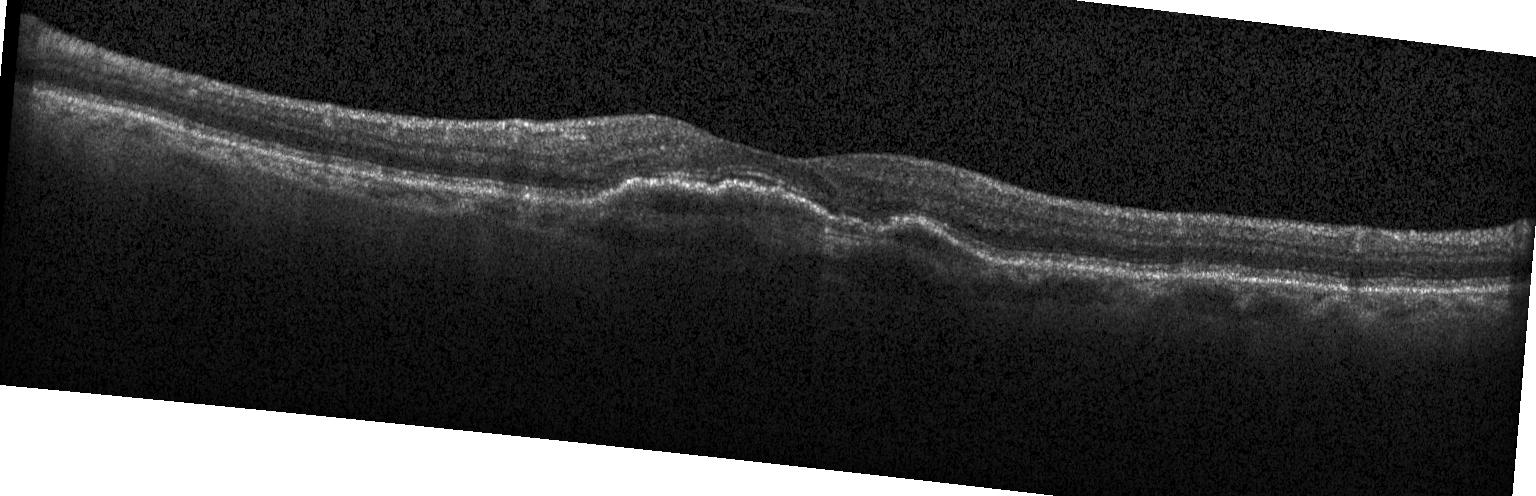 OCT B-scan · SD-OCT.
This B-scan demonstrates a choroidal neovascular membrane.